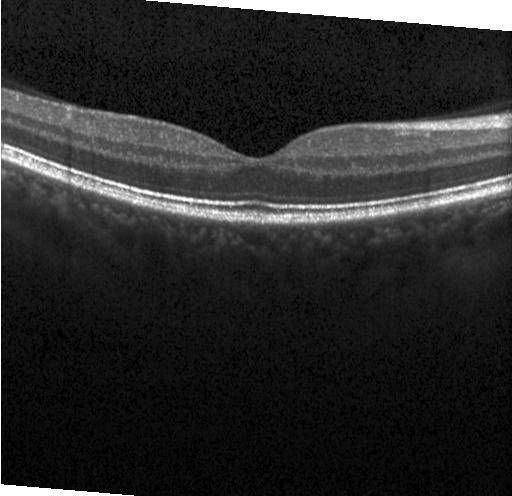

OCT line scan; SD-OCT; instrument: Heidelberg Spectralis; through the macula.
Impression: no evidence of choroidal neovascularization, diabetic macular edema, or drusen.